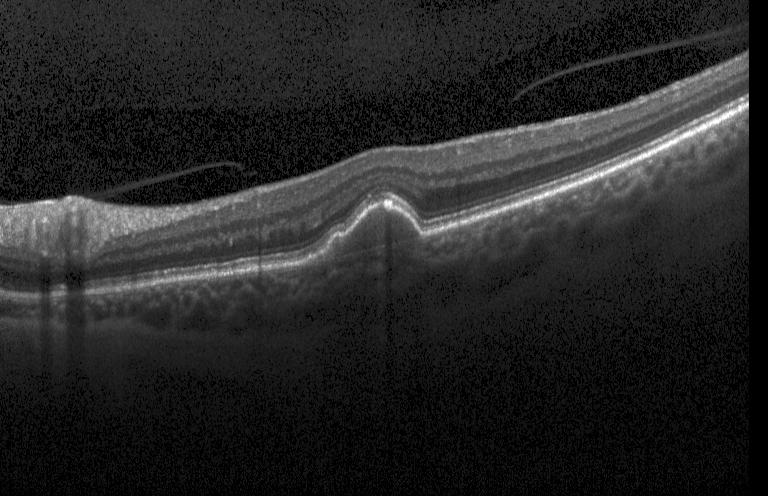

Finding: choroidal neovascularization (CNV).